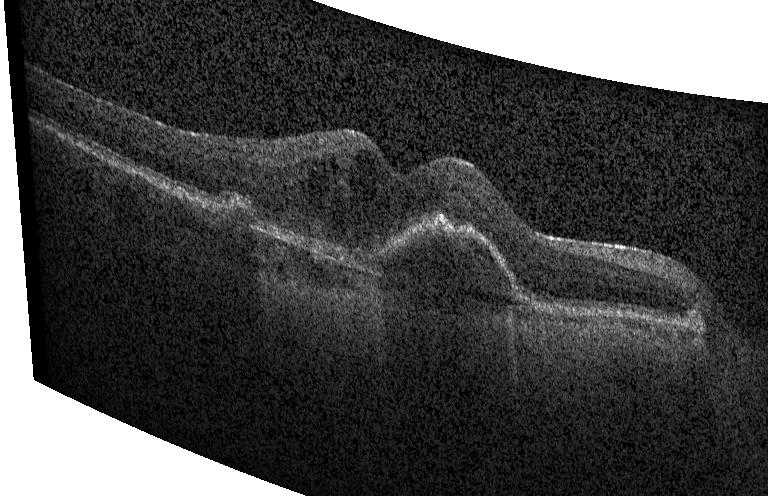
Heidelberg Spectralis. OCT B-scan. Through the macula — Impression: choroidal neovascularization.